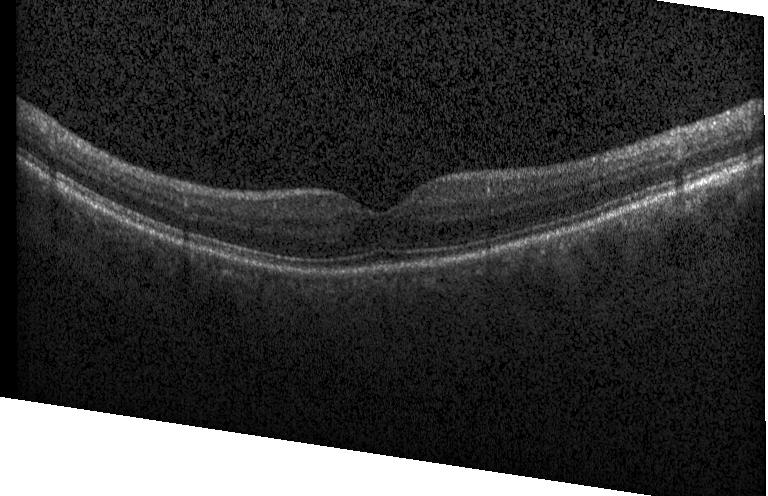 SD-OCT. Optical coherence tomography scan
Impression: neither choroidal neovascularization, diabetic macular edema, nor drusen.